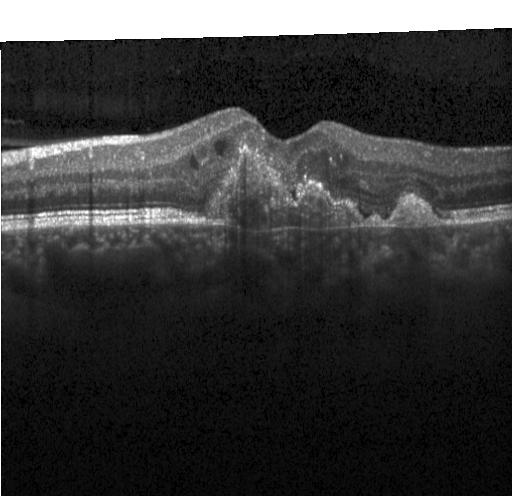

Optical coherence tomography B-scan · acquired on a Heidelberg Spectralis · SD-OCT · fovea-centered.
OCT finding: a choroidal neovascular membrane.